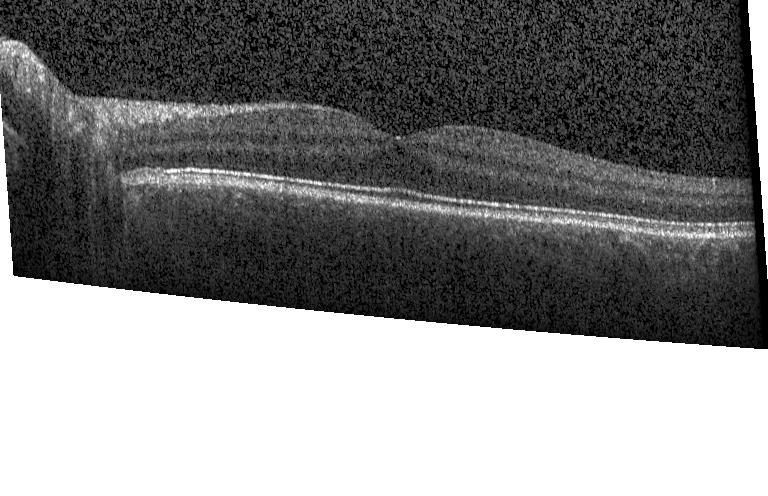

OCT B-scan · acquired on a Heidelberg Spectralis.
The scan shows no choroidal neovascularization, no diabetic macular edema, and no drusen.